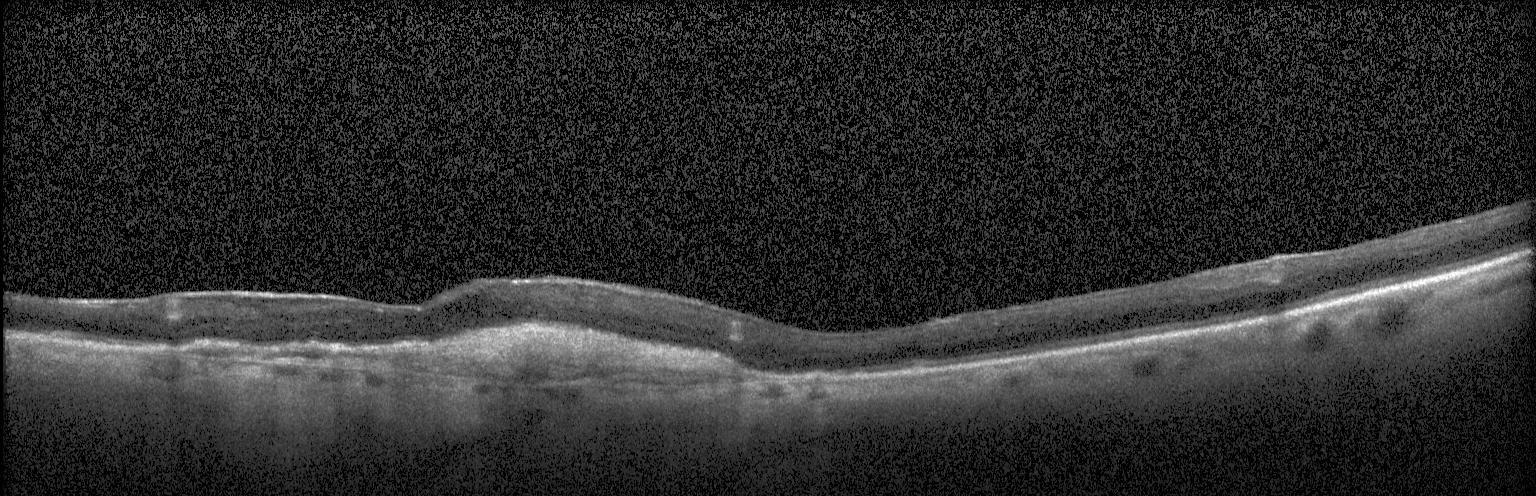
Macular OCT: a choroidal neovascular membrane.